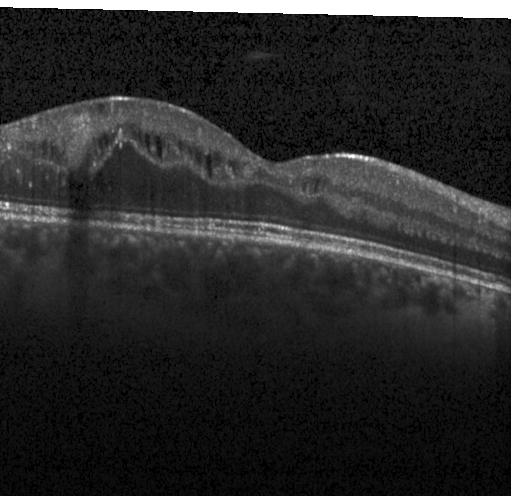

Acquired on a Heidelberg Spectralis; retinal OCT B-scan; through the macula; spectral-domain OCT
Impression: DME.